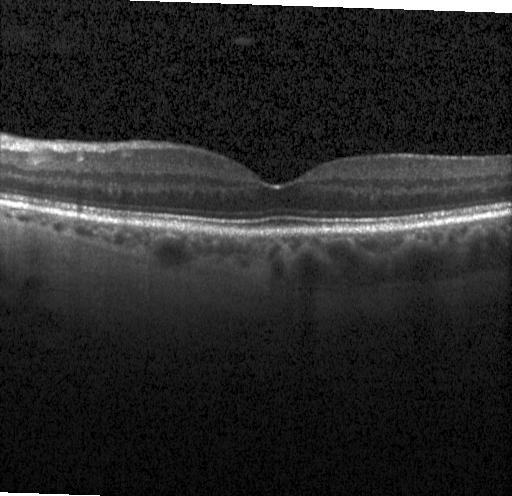

Optical coherence tomography B-scan. Diagnosis: no CNV, no DME, and no drusen.